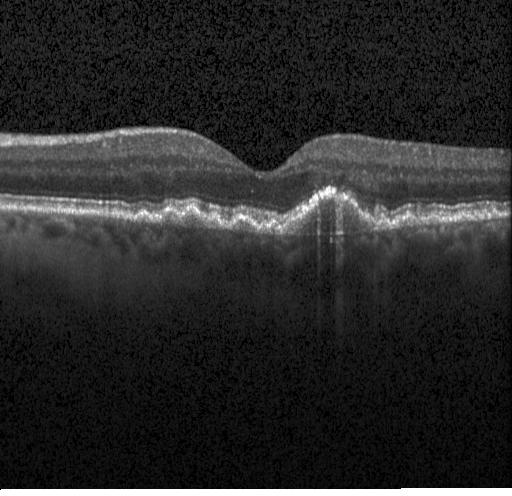

Optical coherence tomography scan, through the macula, acquired on a Heidelberg Spectralis, spectral-domain OCT. Impression: sub-RPE drusenoid deposits.